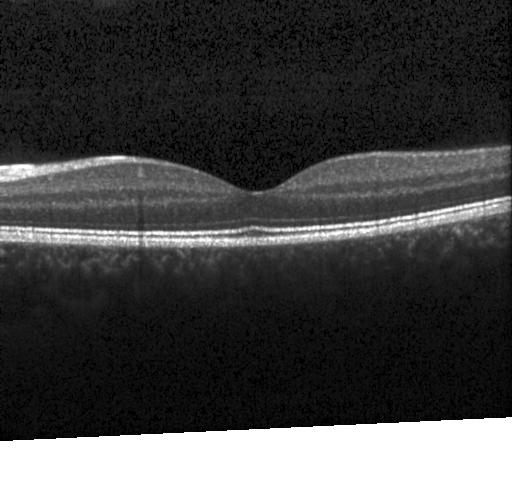
Assessment: no CNV, DME, or drusen.